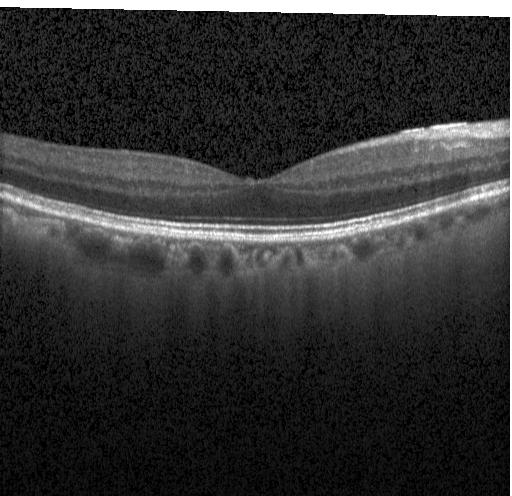

SD-OCT, acquired on a Heidelberg Spectralis, OCT B-scan
Dx: no evidence of choroidal neovascularization, diabetic macular edema, or drusen.